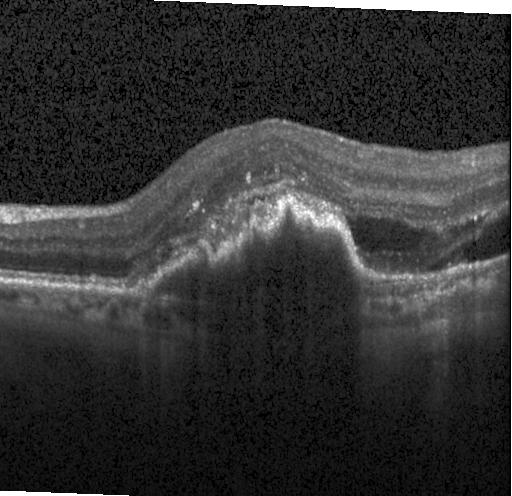
Optical coherence tomography B-scan. SD-OCT. Heidelberg Spectralis — Impression: a choroidal neovascular membrane.